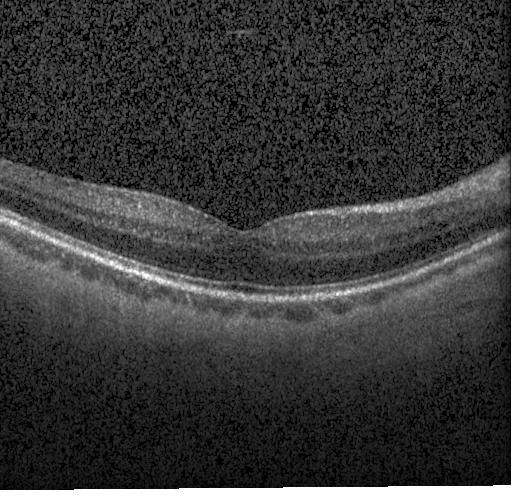

Optical coherence tomography B-scan. Acquired on a Heidelberg Spectralis. Horizontal scan through the fovea
Diagnosis: no choroidal neovascularization, diabetic macular edema, or drusen.